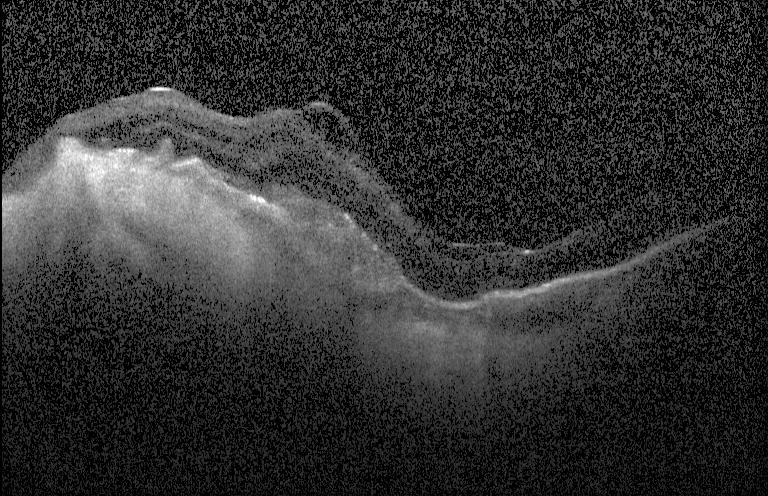 OCT B-scan showing a choroidal neovascular membrane.